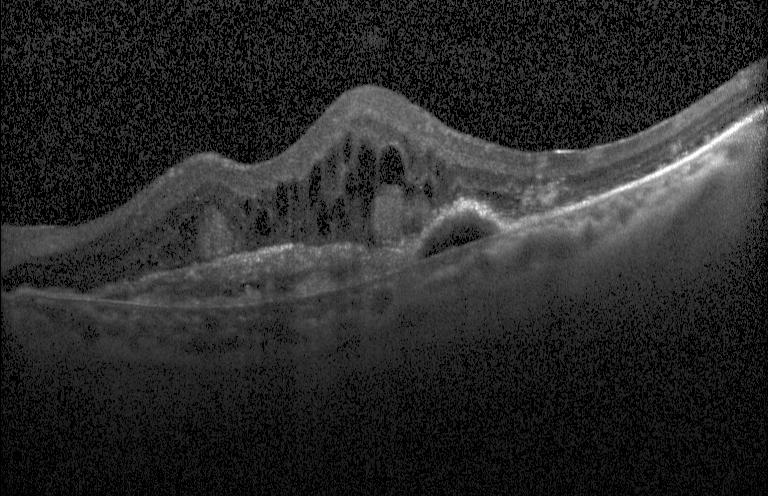 The scan shows choroidal neovascularization.